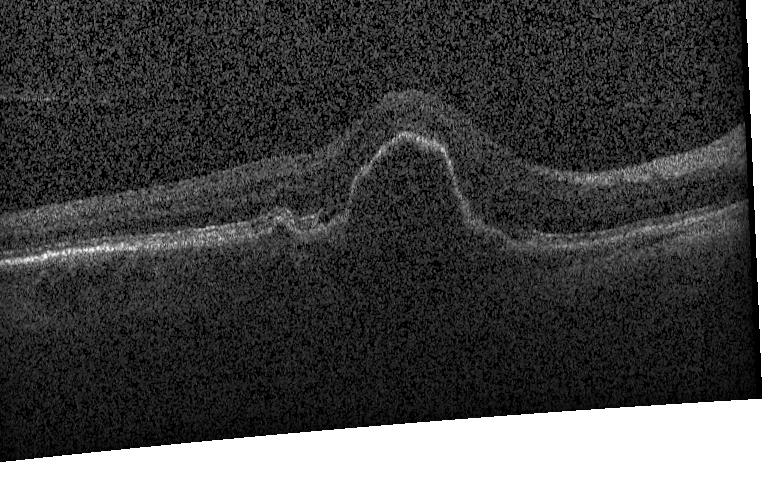

Finding: a choroidal neovascular membrane.